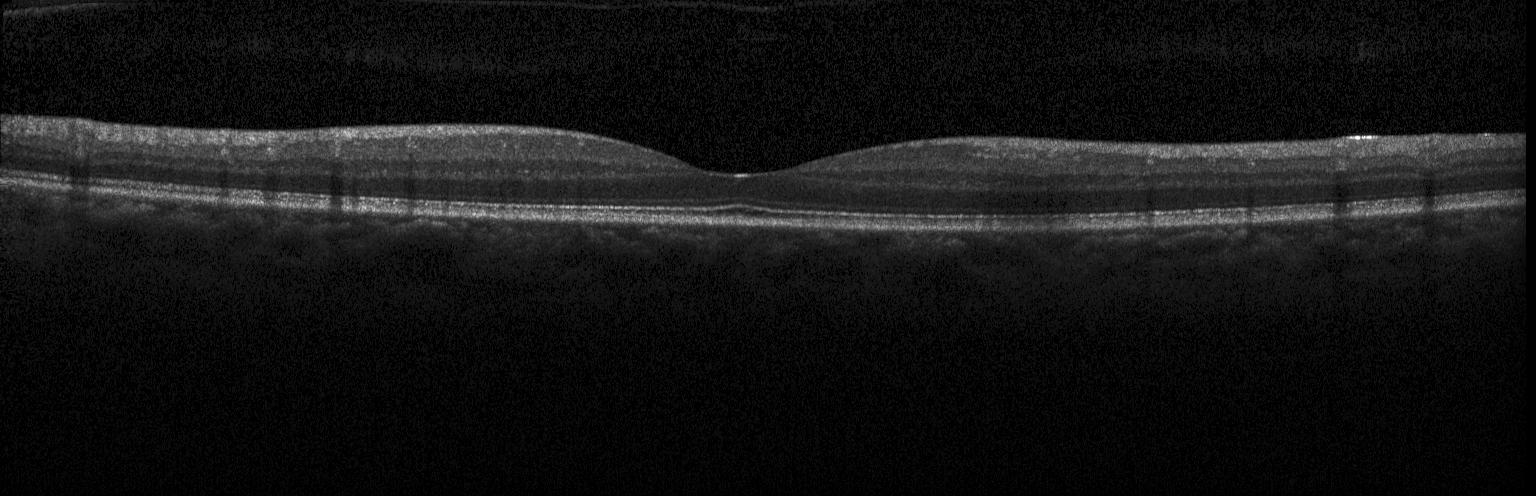 Spectral-domain OCT, retinal OCT cross-section, centered on the fovea
Impression: no choroidal neovascularization, no diabetic macular edema, and no drusen.